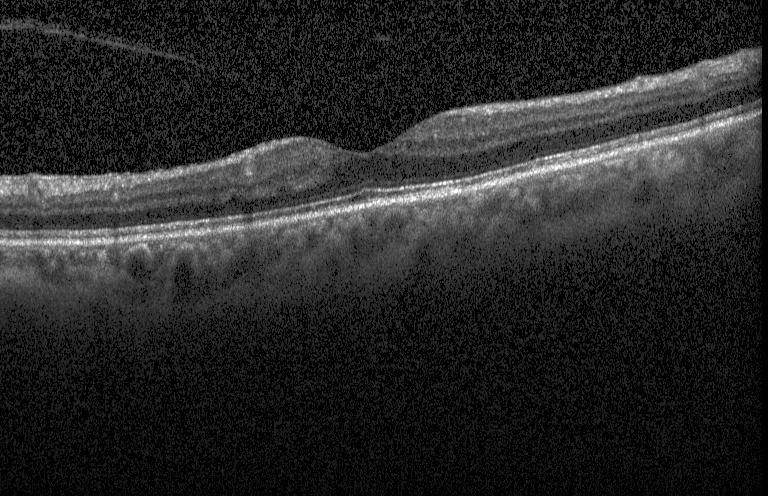 OCT B-scan. Finding: no choroidal neovascularization, diabetic macular edema, or drusen.